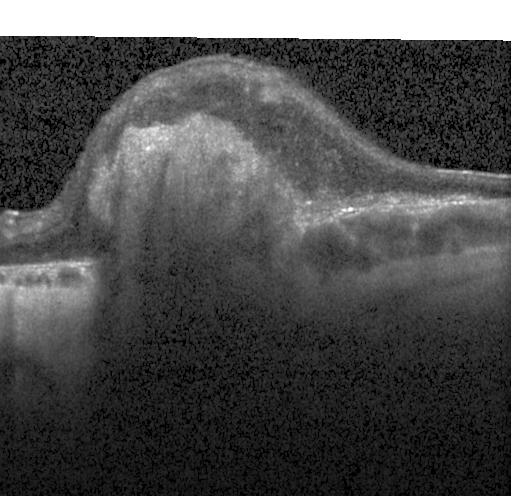 Impression: a choroidal neovascular membrane.